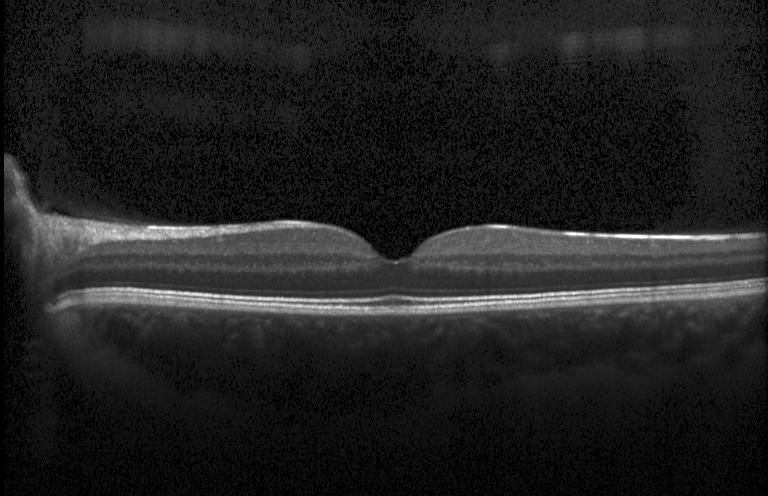 Retinal OCT cross-section showing no evidence of choroidal neovascularization, diabetic macular edema, or drusen.